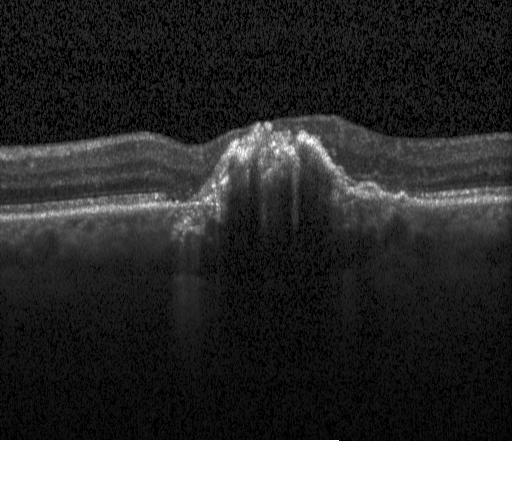 A choroidal neovascular membrane.